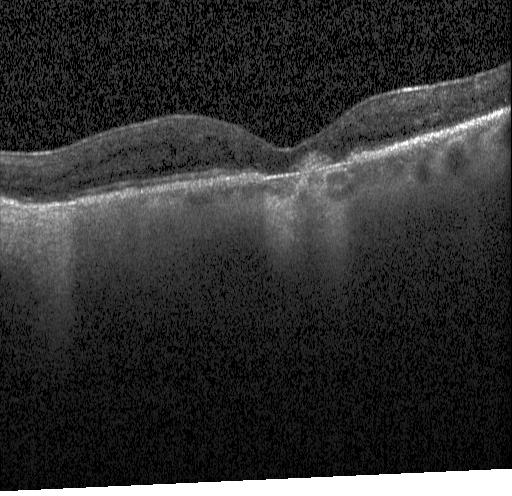

OCT line scan — Impression: CNV.